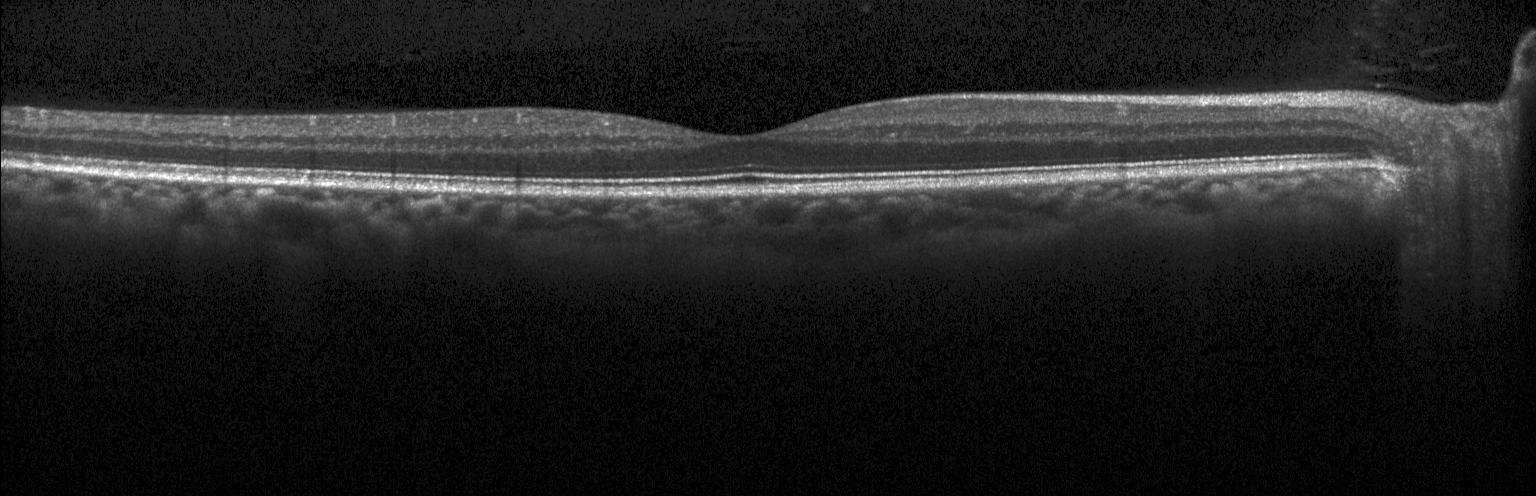
Horizontal scan through the fovea. Optical coherence tomography B-scan
Macular OCT: no evidence of choroidal neovascularization, diabetic macular edema, or drusen.